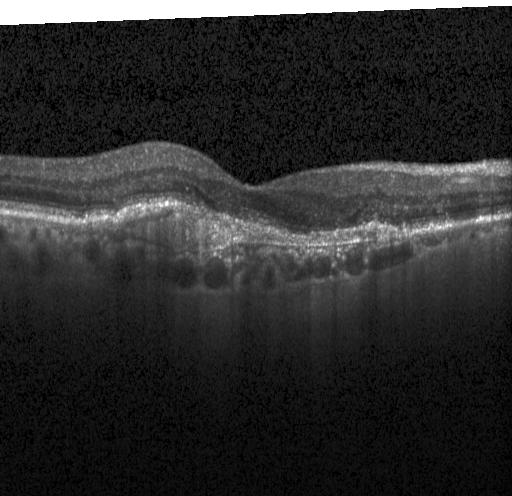

OCT finding: a choroidal neovascular membrane.